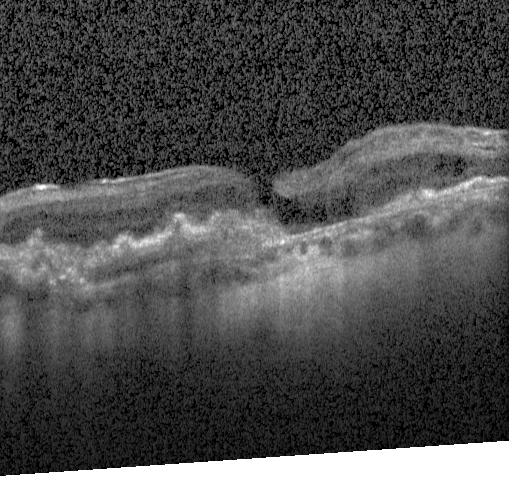

Optical coherence tomography B-scan — This B-scan demonstrates a choroidal neovascular membrane.